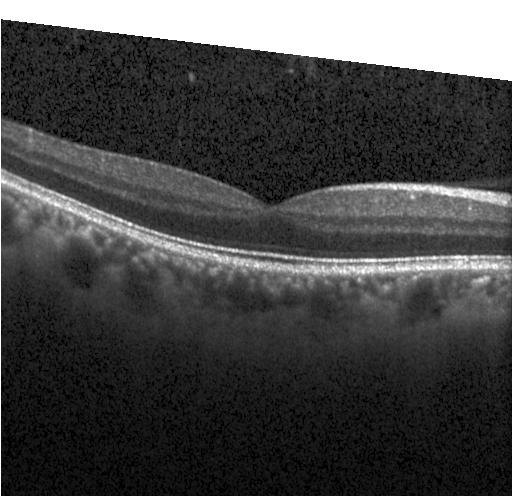

The scan shows no choroidal neovascularization, diabetic macular edema, or drusen.